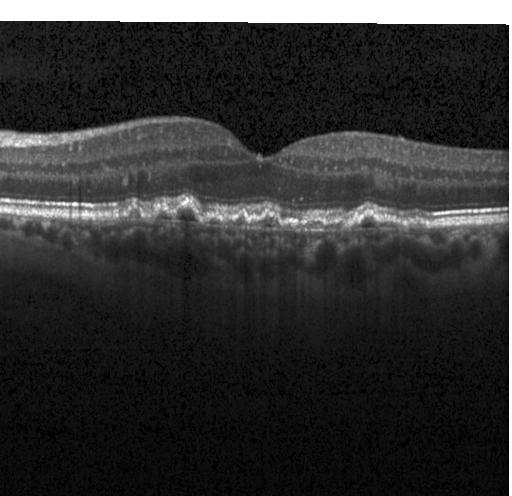

Optical coherence tomography B-scan · instrument: Heidelberg Spectralis — OCT finding: sub-RPE drusenoid deposits.